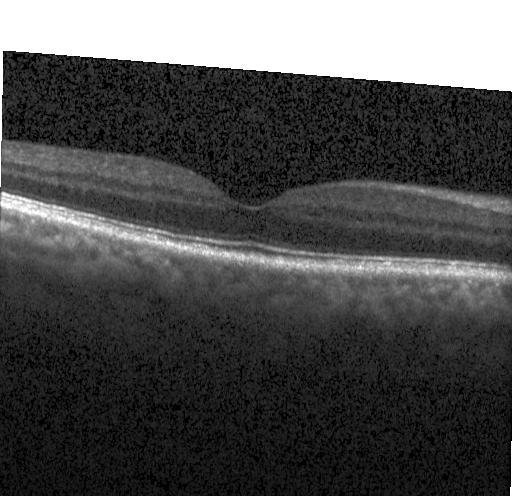
SD-OCT. Retinal OCT B-scan — The scan shows no choroidal neovascularization, diabetic macular edema, or drusen.